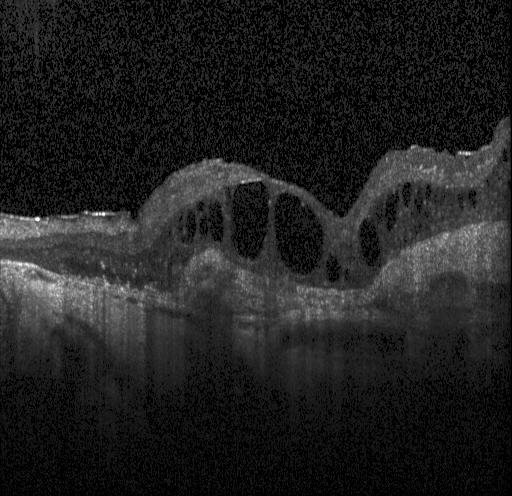 Assessment: a choroidal neovascular membrane.